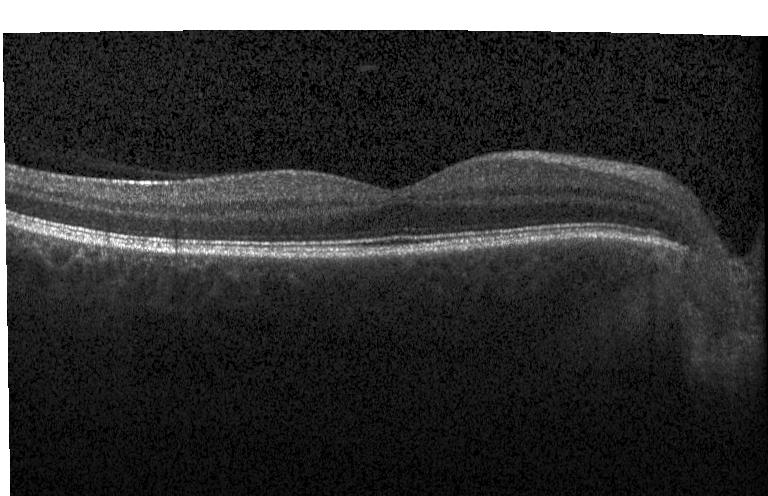

Retinal OCT cross-section · Heidelberg Spectralis OCT system · SD-OCT. Assessment: no CNV, no DME, and no drusen.